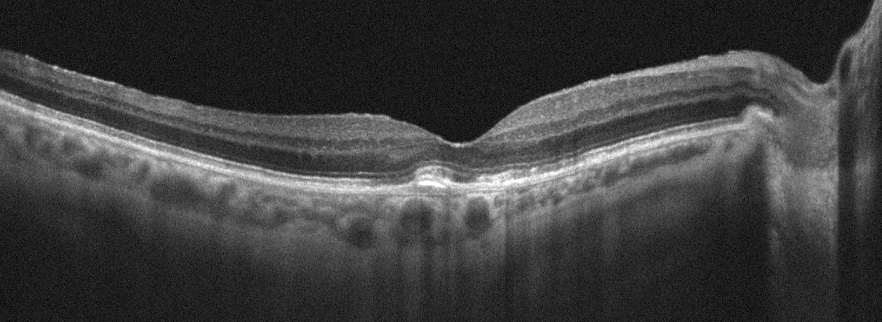 OCT B-scan; macular scan; instrument: Optovue Avanti RTVue XR — Macular OCT: age-related macular degeneration (AMD).